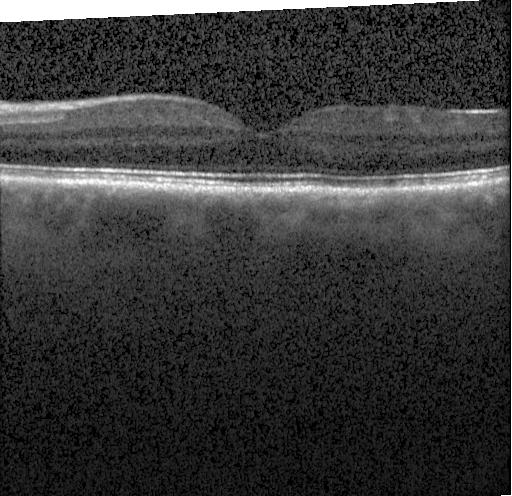
Optical coherence tomography B-scan · SD-OCT · acquired on a Heidelberg Spectralis · fovea-centered
Impression: no CNV, DME, or drusen.